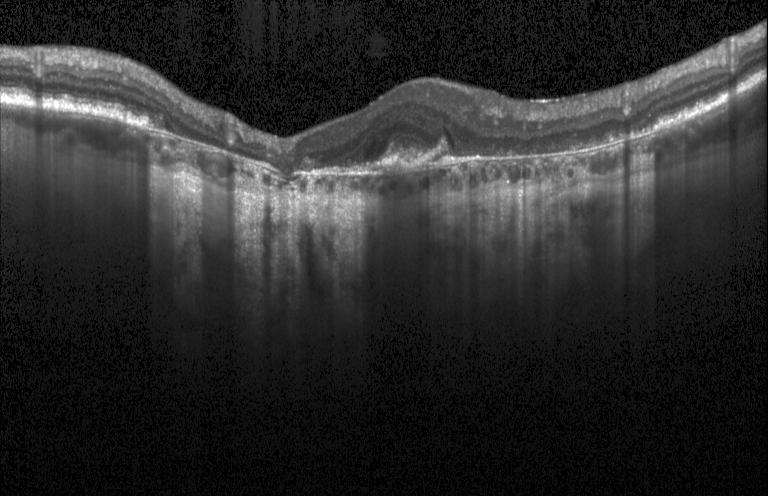

Optical coherence tomography B-scan, Heidelberg Spectralis OCT system, centered on the fovea. Choroidal neovascularization (CNV).